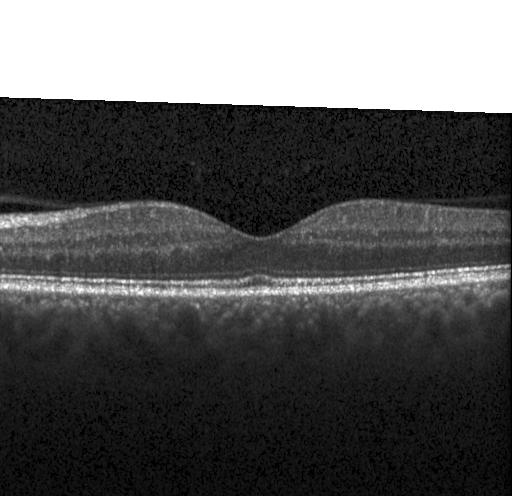 Retinal OCT cross-section. Spectral-domain optical coherence tomography. Heidelberg Spectralis. Fovea-centered
Neither choroidal neovascularization, diabetic macular edema, nor drusen.